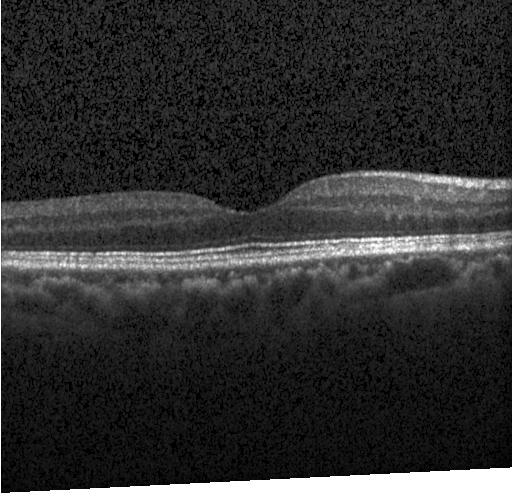

SD-OCT, optical coherence tomography B-scan, macular scan — This B-scan demonstrates no choroidal neovascularization, no diabetic macular edema, and no drusen.